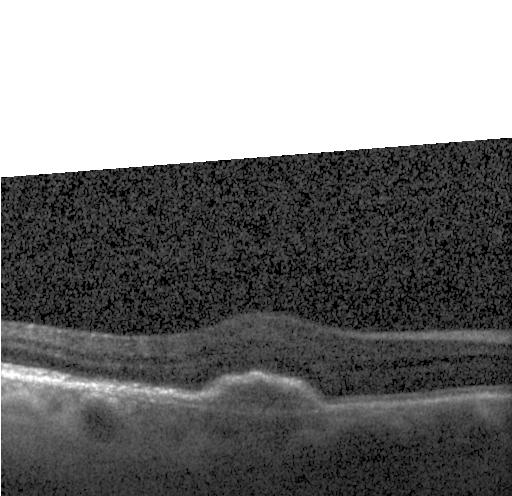 Spectral-domain optical coherence tomography, through the macula, retinal OCT cross-section. Macular OCT: a choroidal neovascular membrane.